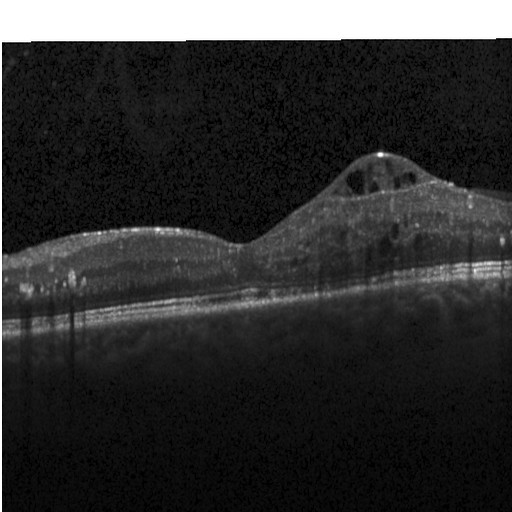 Diagnosis: diabetic macular edema (DME).